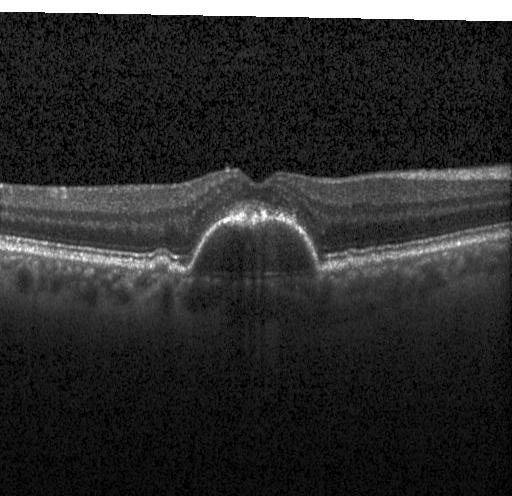
Impression: CNV.